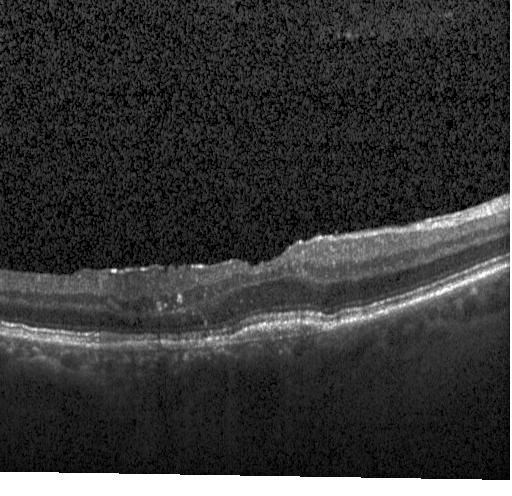

OCT finding: a choroidal neovascular membrane.